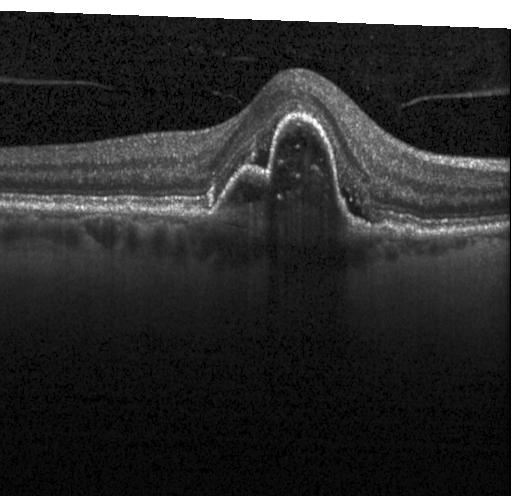

Finding: a choroidal neovascular membrane.